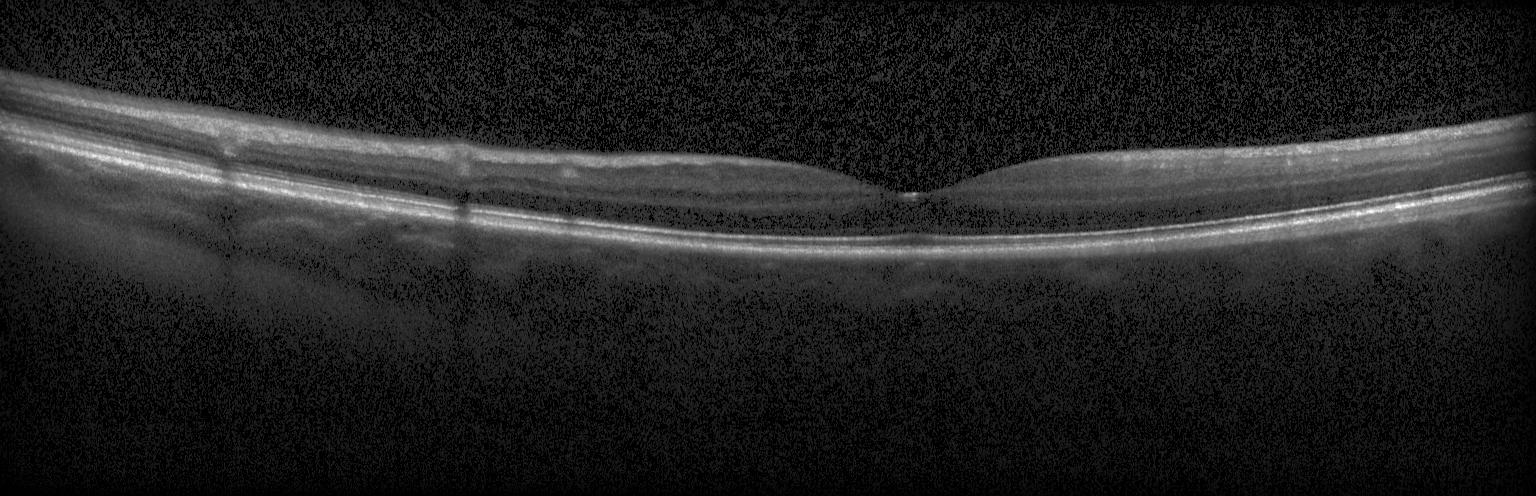
OCT B-scan — Impression: no evidence of choroidal neovascularization, diabetic macular edema, or drusen.